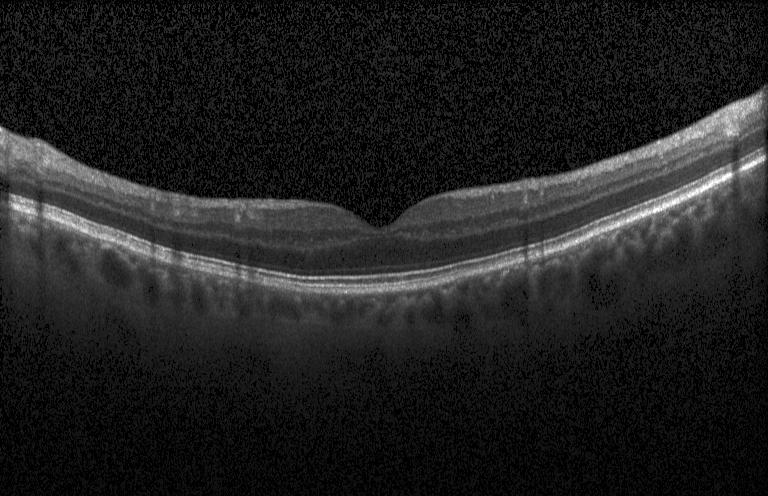

Optical coherence tomography B-scan.
This B-scan demonstrates neither choroidal neovascularization, diabetic macular edema, nor drusen.